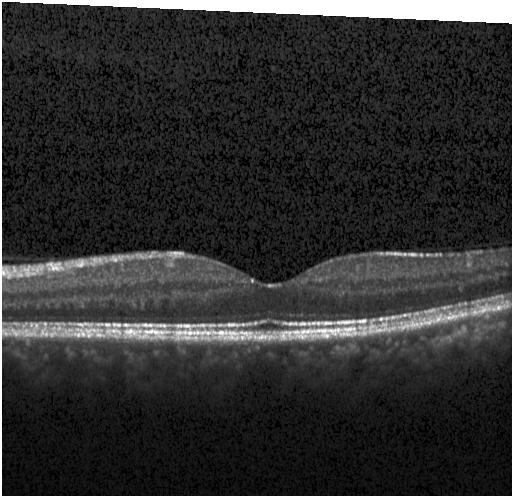

This B-scan demonstrates neither CNV, DME, nor drusen.